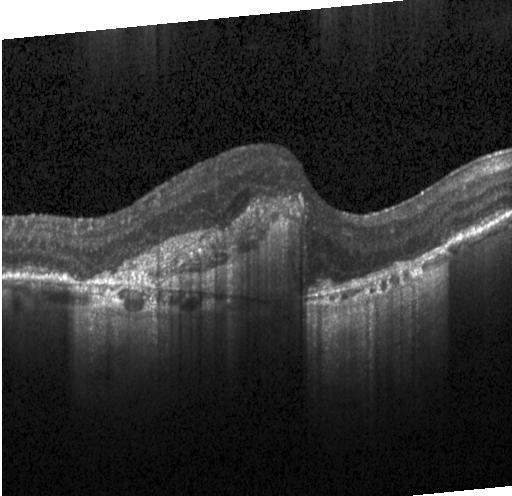 OCT line scan. Impression: choroidal neovascularization (CNV).